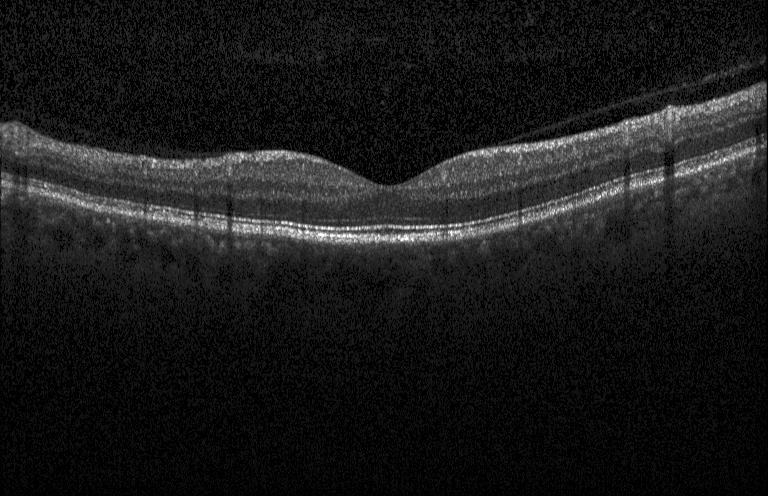 Finding: neither choroidal neovascularization, diabetic macular edema, nor drusen.